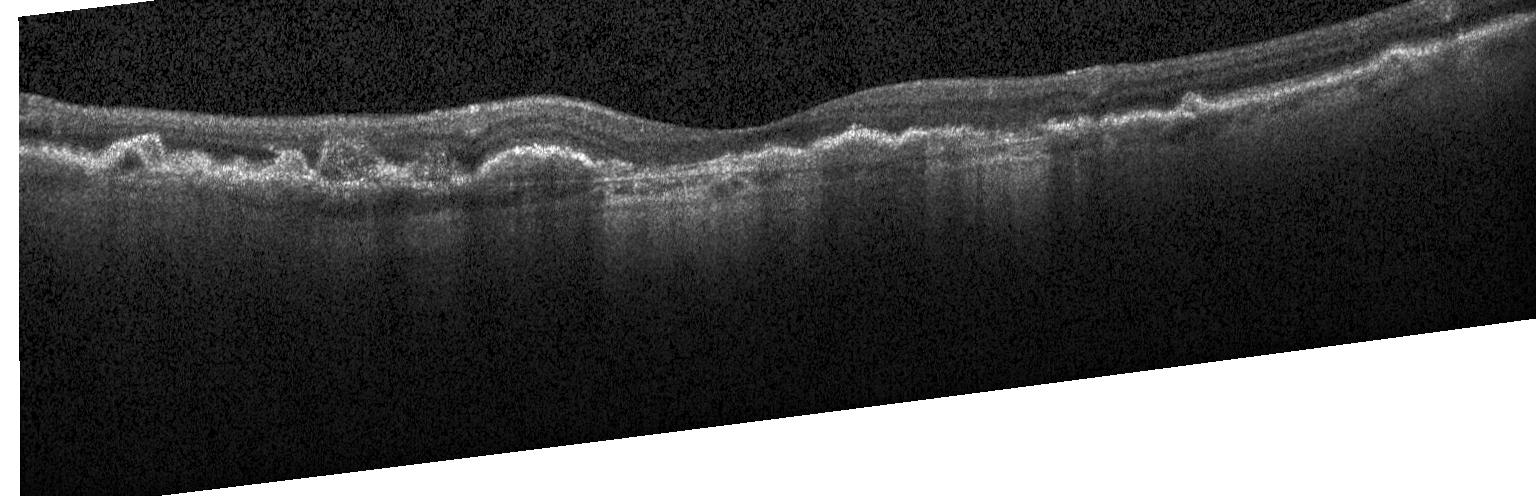
Macular OCT: a choroidal neovascular membrane.